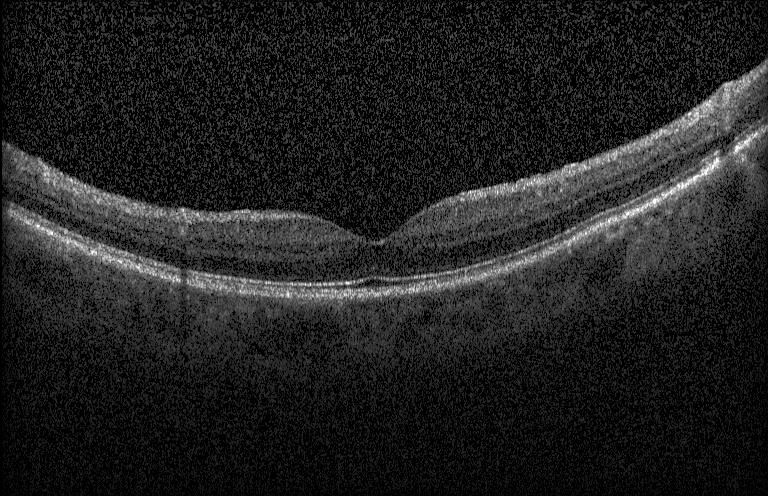

Diagnosis: no CNV, DME, or drusen.